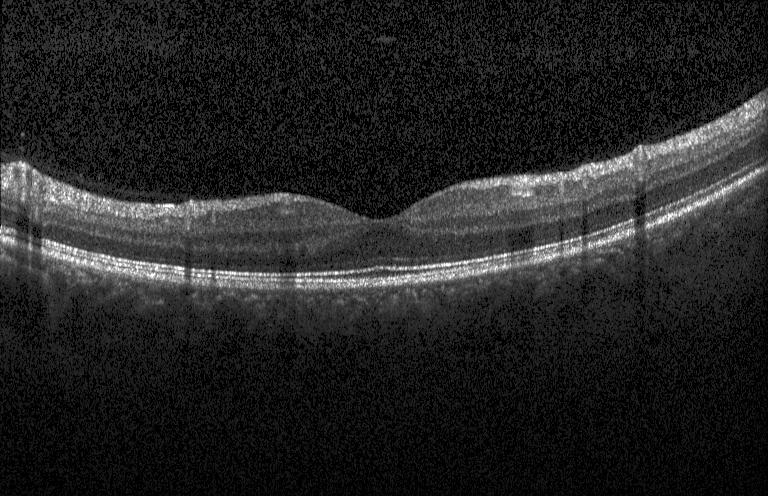
Diagnosis: no evidence of CNV, DME, or drusen.